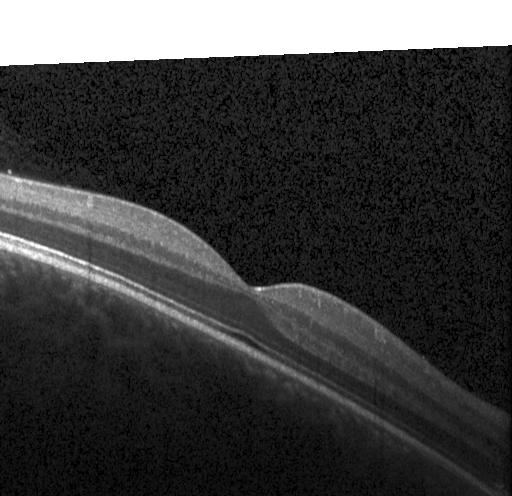 Horizontal scan through the fovea · Heidelberg Spectralis · spectral-domain optical coherence tomography · OCT B-scan
Assessment: no CNV, no DME, and no drusen.